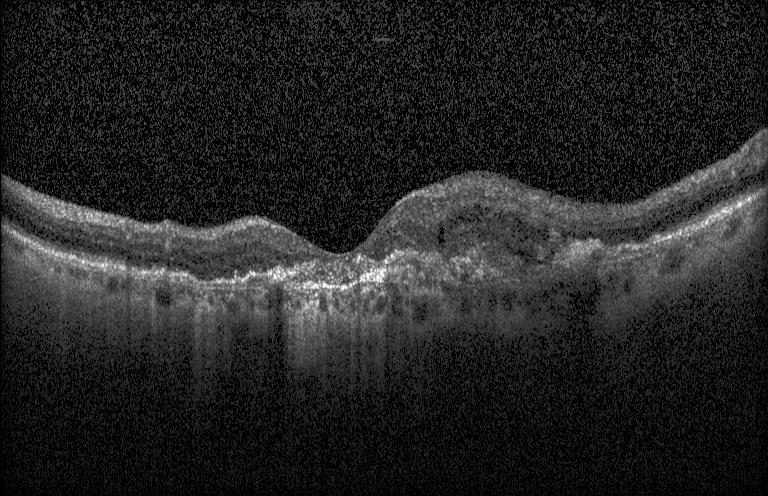 Acquired on a Heidelberg Spectralis. Retinal OCT B-scan. OCT finding: choroidal neovascularization (CNV).